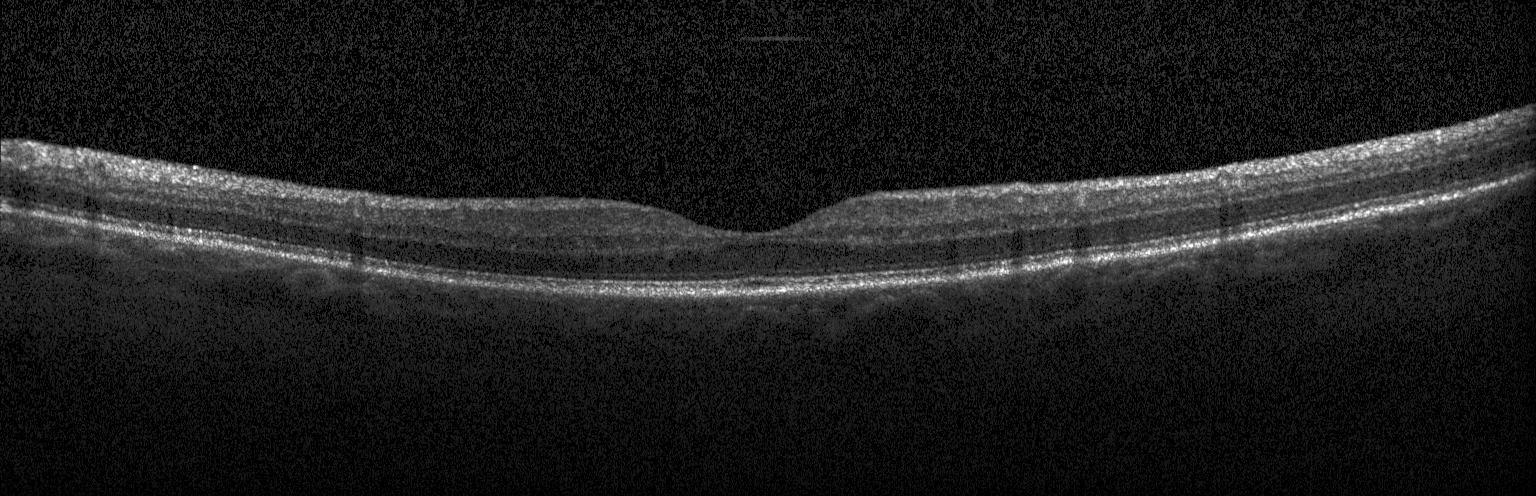 Assessment: no choroidal neovascularization, diabetic macular edema, or drusen.